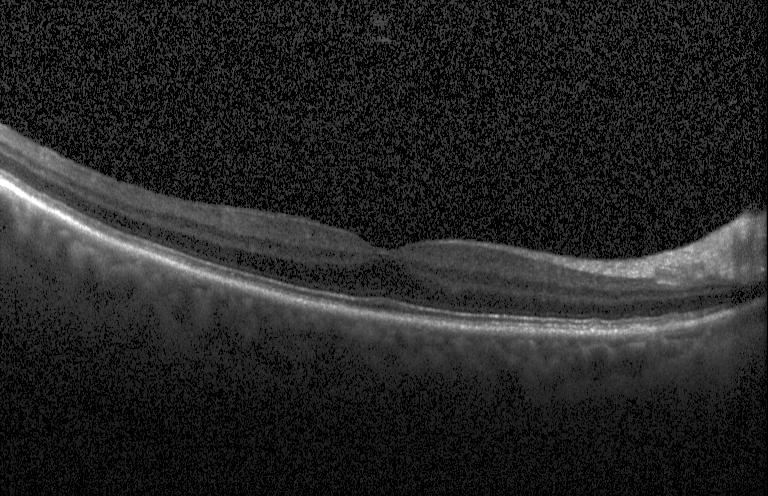

Finding: no choroidal neovascularization, no diabetic macular edema, and no drusen.